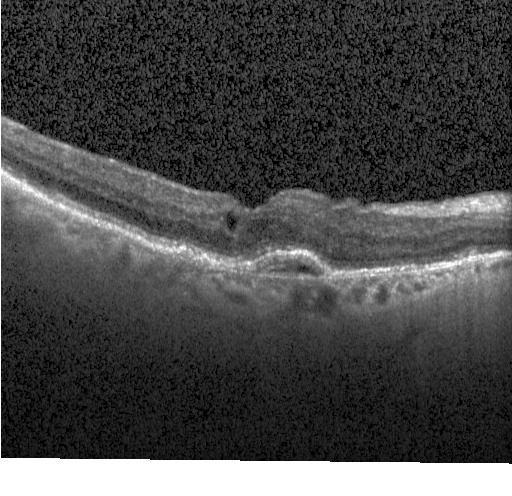

Retinal OCT cross-section, acquired on a Heidelberg Spectralis.
Dx: a choroidal neovascular membrane.